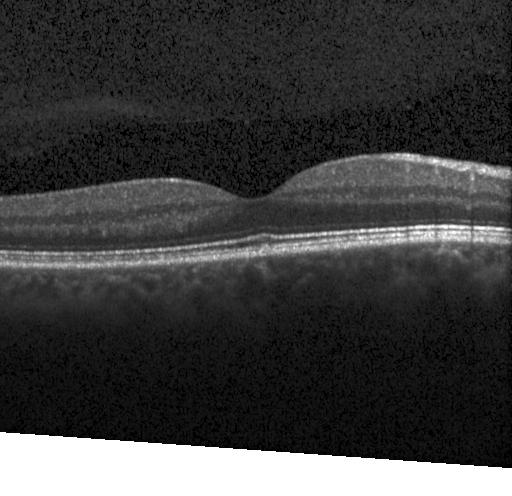
Retinal OCT cross-section; SD-OCT.
Diagnosis: no CNV, DME, or drusen.